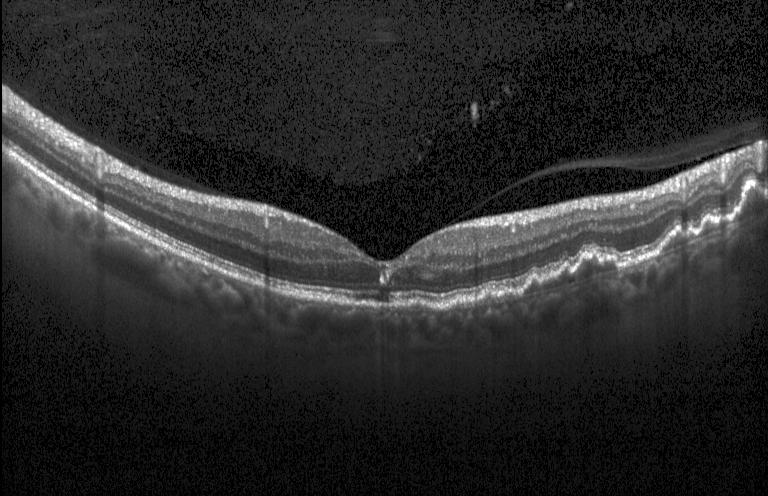
Macular scan; acquired on a Heidelberg Spectralis; optical coherence tomography scan
Finding: a choroidal neovascular membrane.